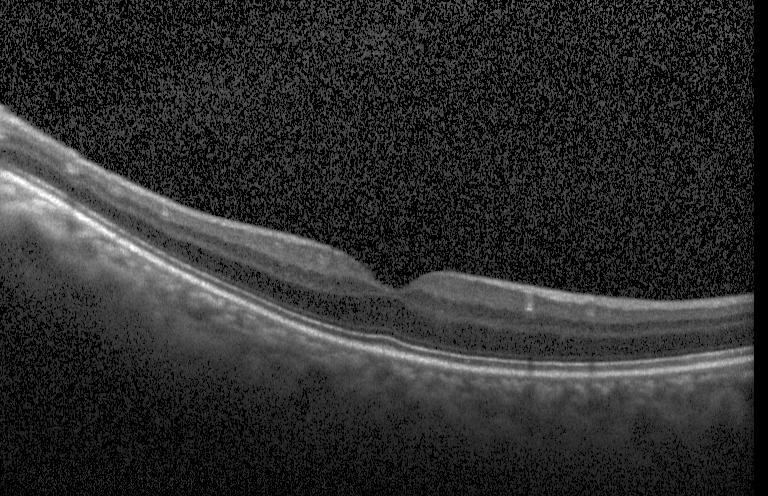 Through the macula; retinal OCT cross-section; spectral-domain OCT.
This B-scan demonstrates no evidence of CNV, DME, or drusen.